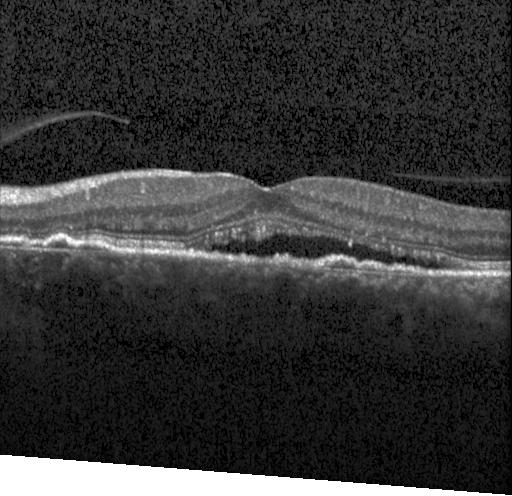 Retinal OCT cross-section
Finding: a choroidal neovascular membrane.